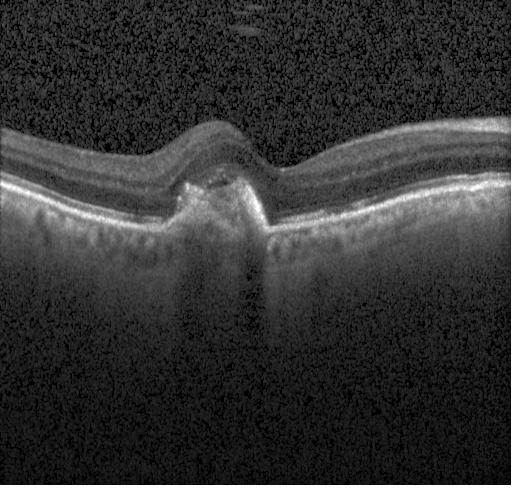

Retinal OCT B-scan · instrument: Heidelberg Spectralis · macular scan — Diagnosis: choroidal neovascularization.